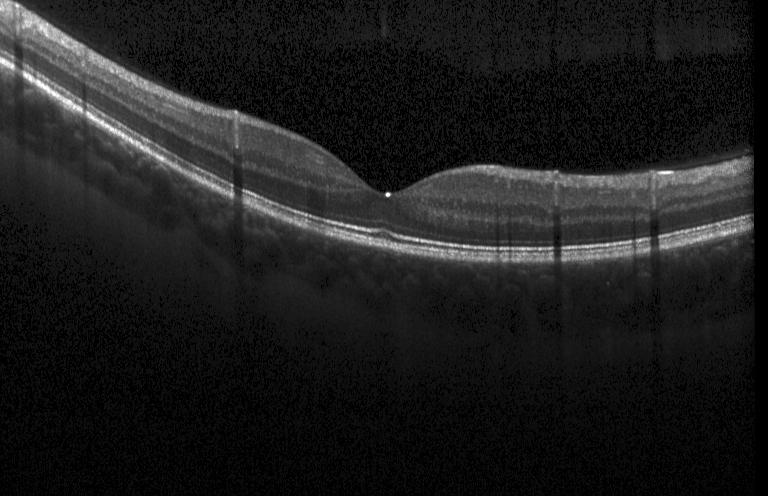
Retinal OCT B-scan
Macular OCT: no CNV, DME, or drusen.